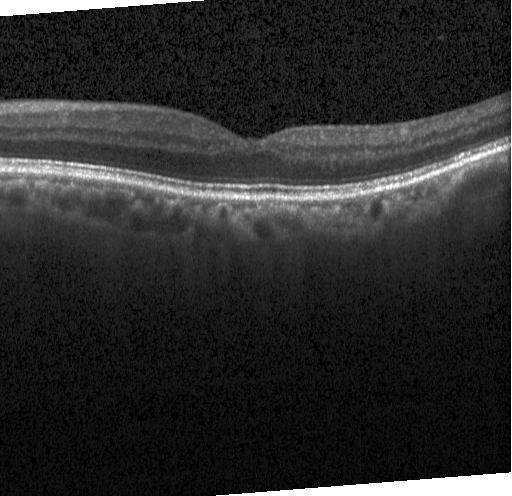

OCT B-scan — No evidence of choroidal neovascularization, diabetic macular edema, or drusen.